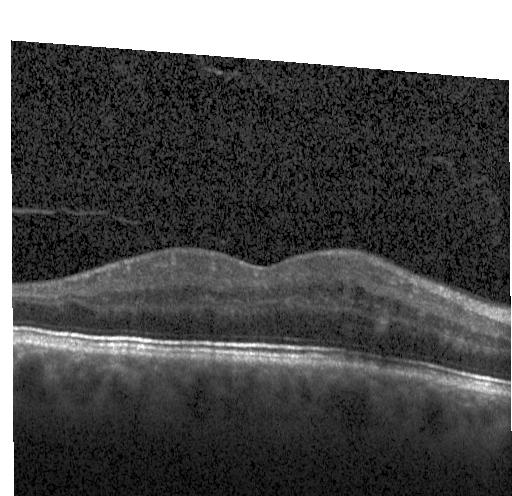

Impression: diabetic macular edema (DME).